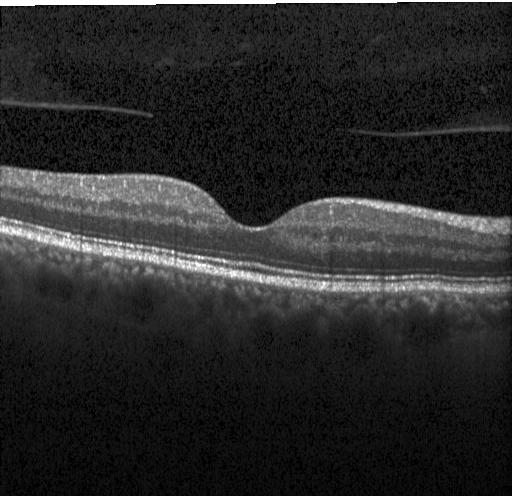

Fovea-centered; OCT line scan — Neither choroidal neovascularization, diabetic macular edema, nor drusen.